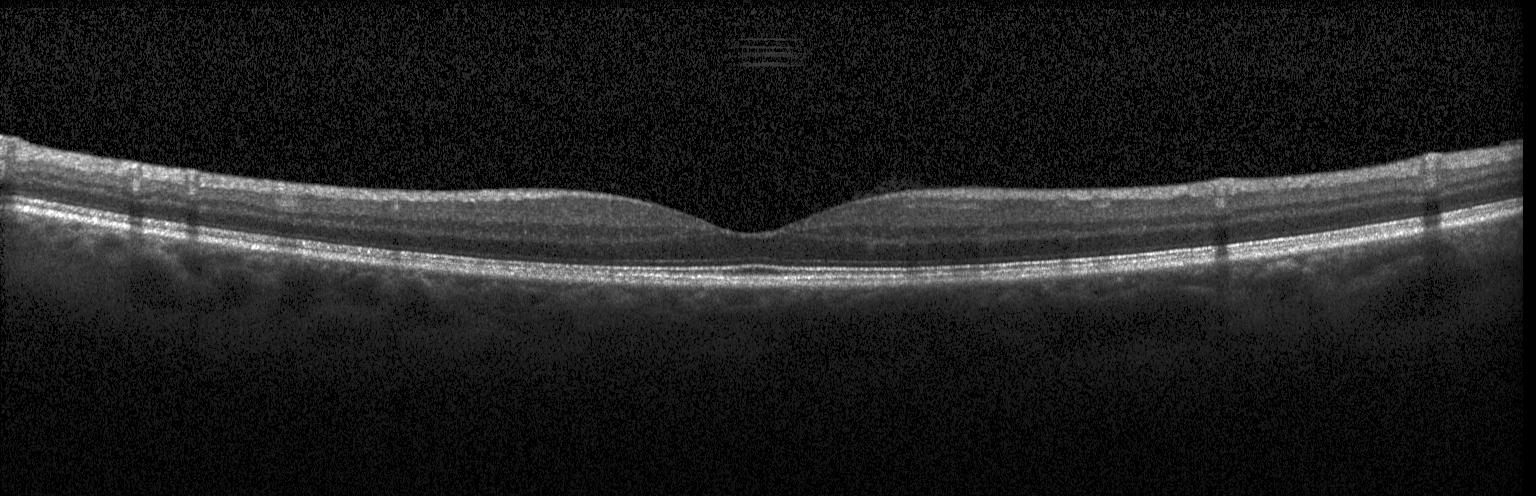 Diagnosis: neither choroidal neovascularization, diabetic macular edema, nor drusen.